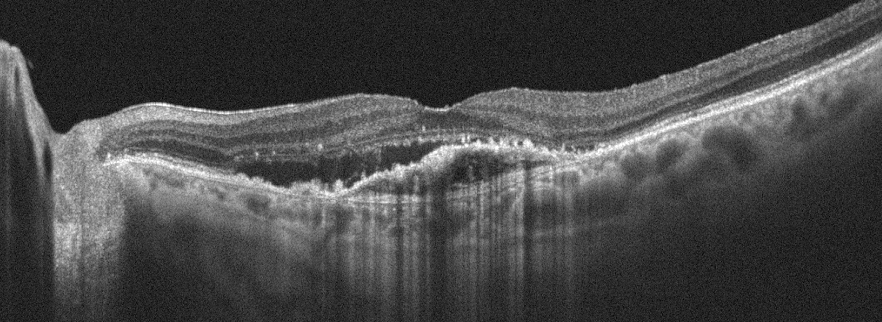

OCT B-scan. Left eye
OCT finding: age-related macular degeneration (AMD).